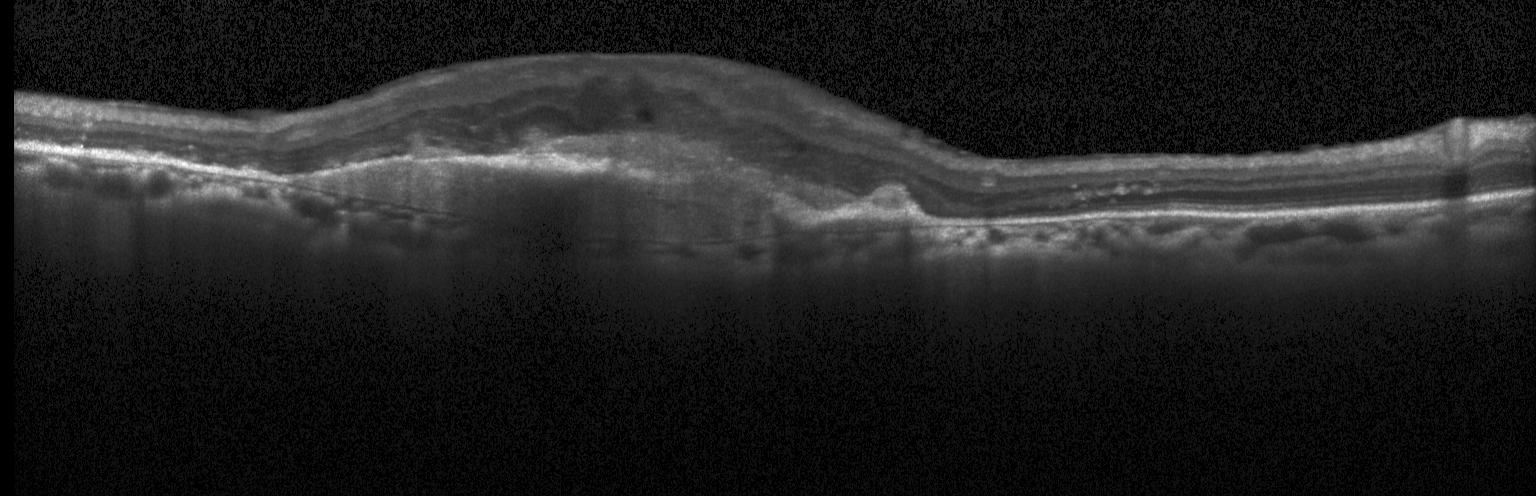
Finding: choroidal neovascularization.